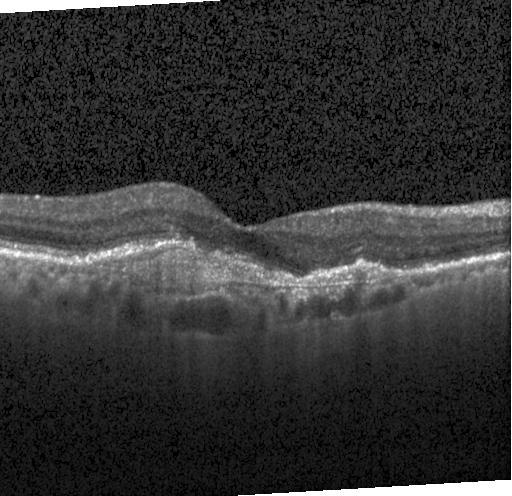

Macular OCT demonstrating choroidal neovascularization (CNV).